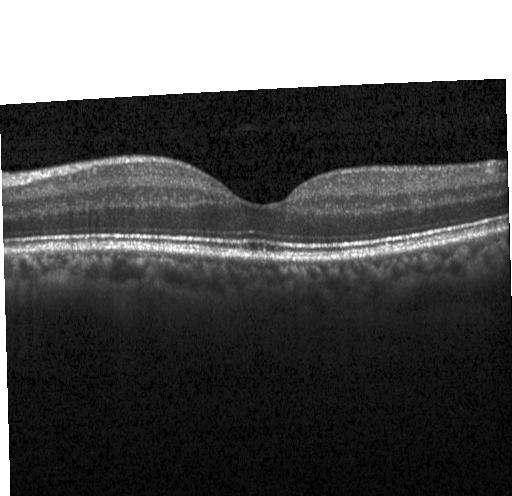

OCT finding: no evidence of CNV, DME, or drusen.